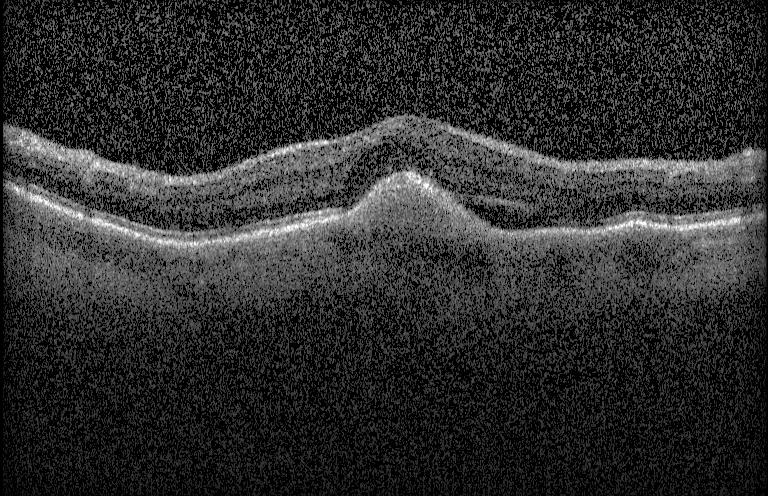 Finding: a choroidal neovascular membrane.